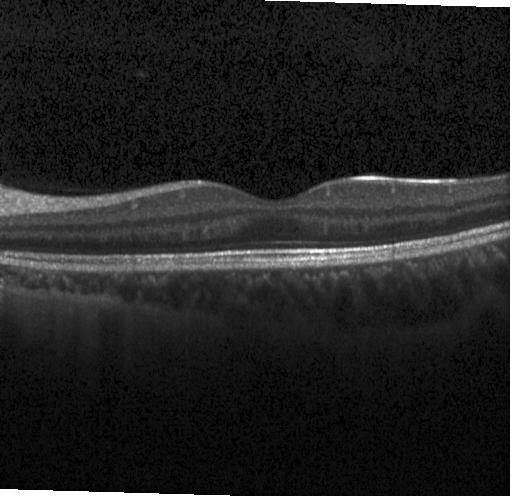 OCT line scan. Diagnosis: no CNV, DME, or drusen.